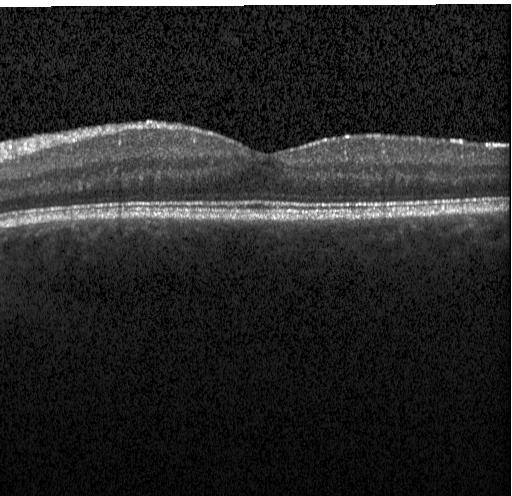
Optical coherence tomography B-scan. Centered on the fovea. Spectral-domain optical coherence tomography — Finding: neither choroidal neovascularization, diabetic macular edema, nor drusen.